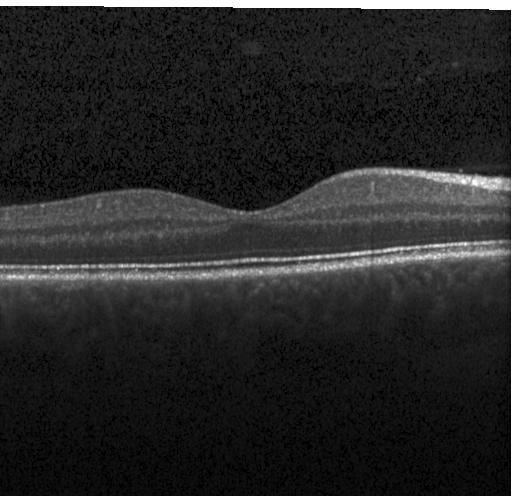

Dx: no choroidal neovascularization, diabetic macular edema, or drusen.